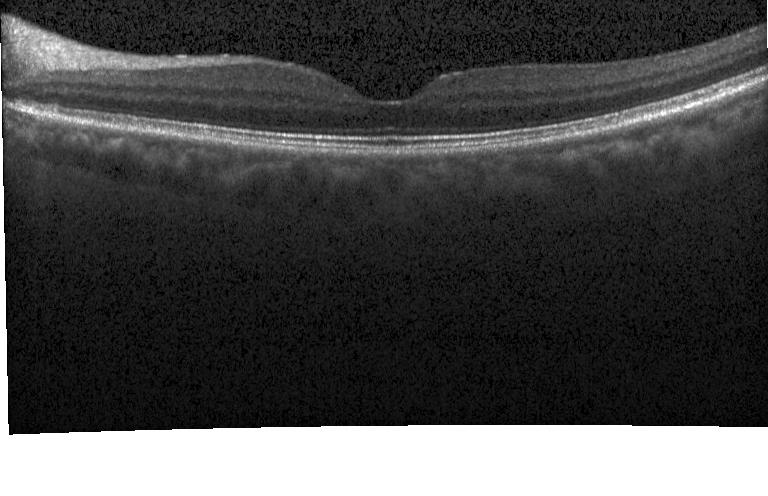

Macular OCT demonstrating neither choroidal neovascularization, diabetic macular edema, nor drusen.